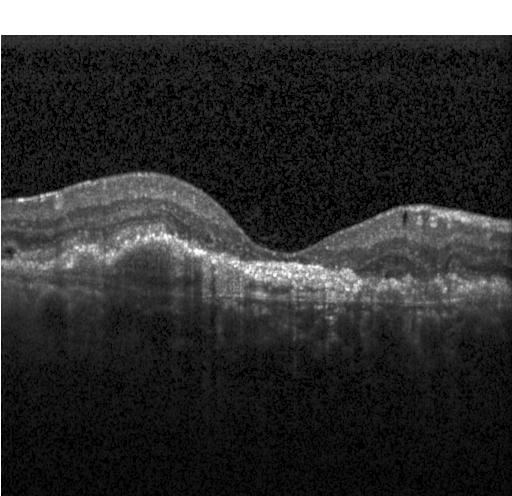

OCT scan showing a choroidal neovascular membrane.